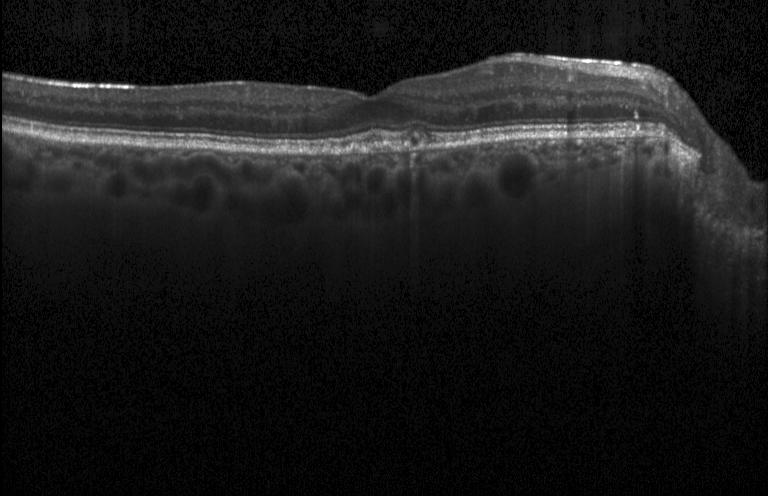

Optical coherence tomography B-scan, instrument: Heidelberg Spectralis.
This B-scan demonstrates drusen.